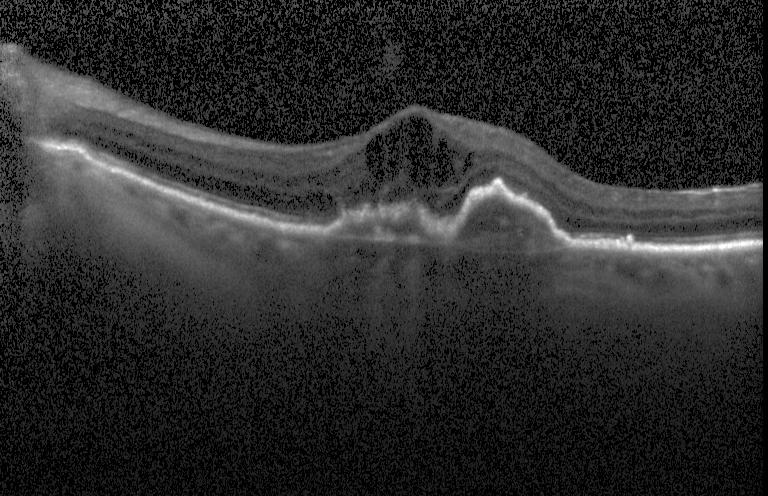 Finding: choroidal neovascularization.